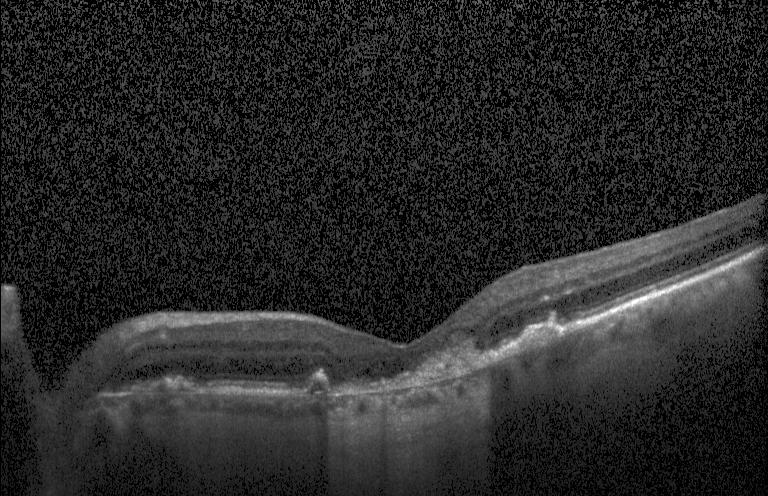 OCT scan showing choroidal neovascularization (CNV).